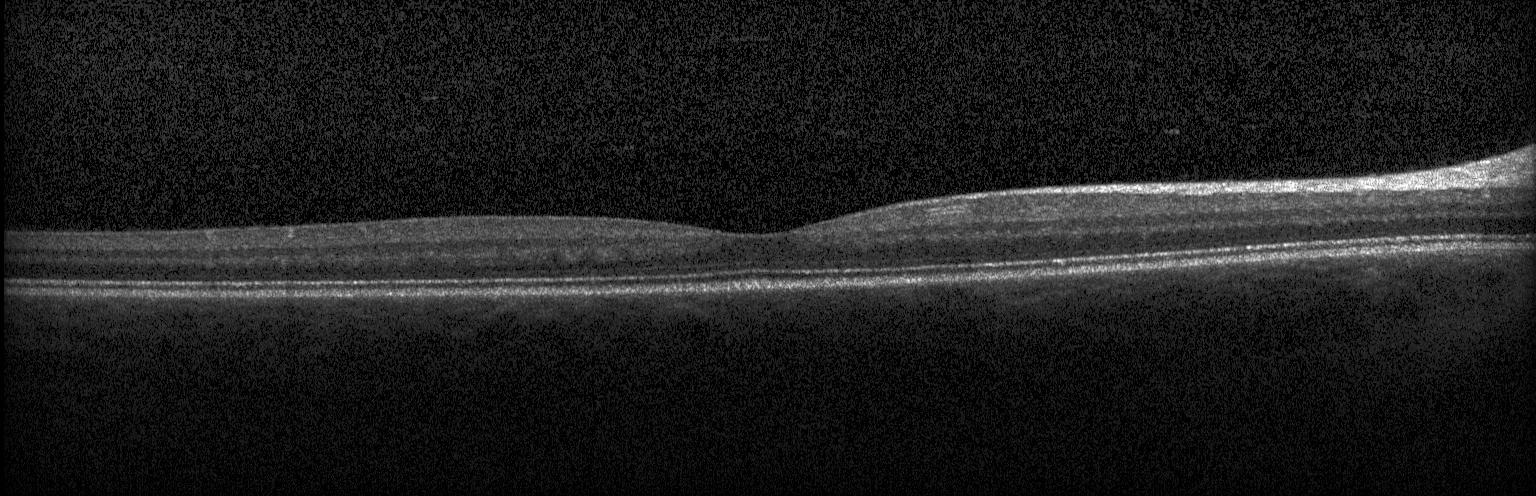

OCT B-scan showing no CNV, DME, or drusen.